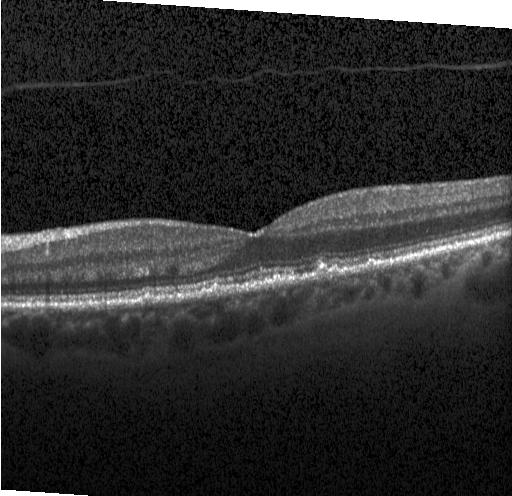 Instrument: Heidelberg Spectralis, through the macula, spectral-domain OCT, retinal OCT B-scan.
Multiple drusen.